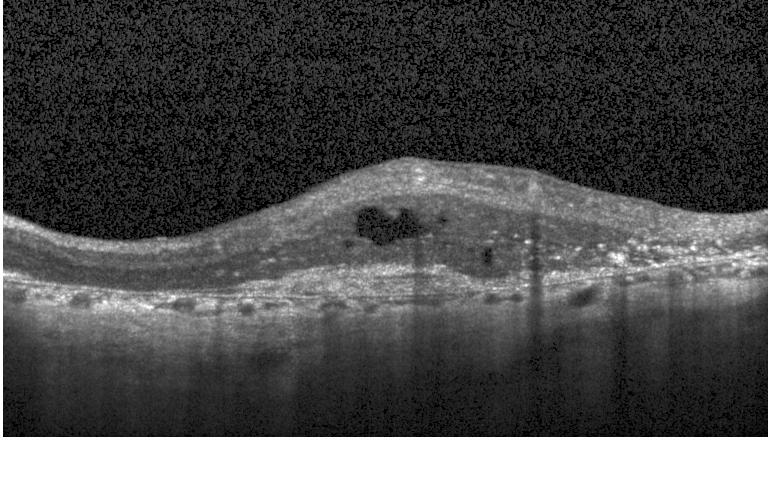 Assessment: choroidal neovascularization (CNV).